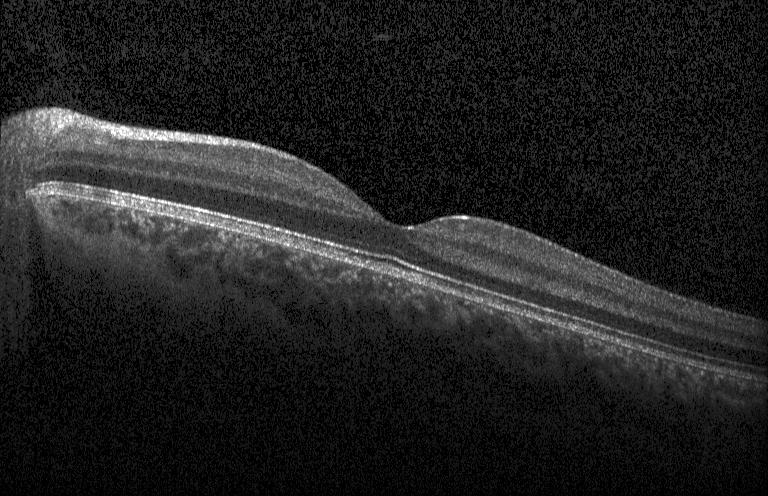

Macular OCT: neither choroidal neovascularization, diabetic macular edema, nor drusen.